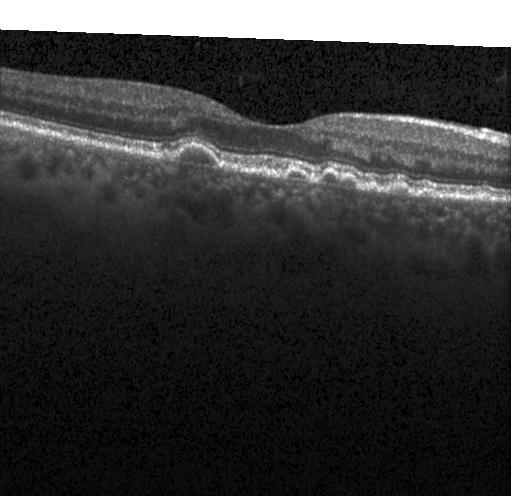 OCT scan showing drusen.